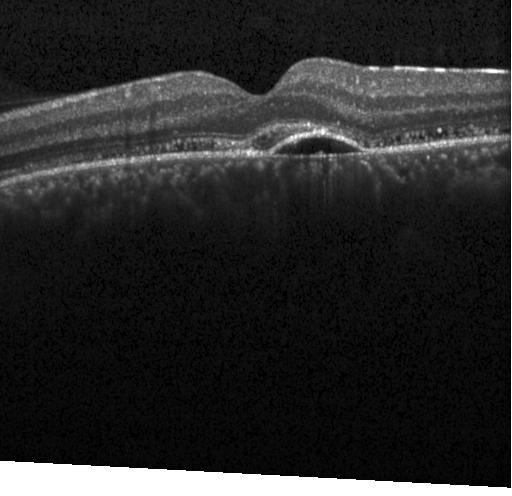
Macular OCT: choroidal neovascularization.